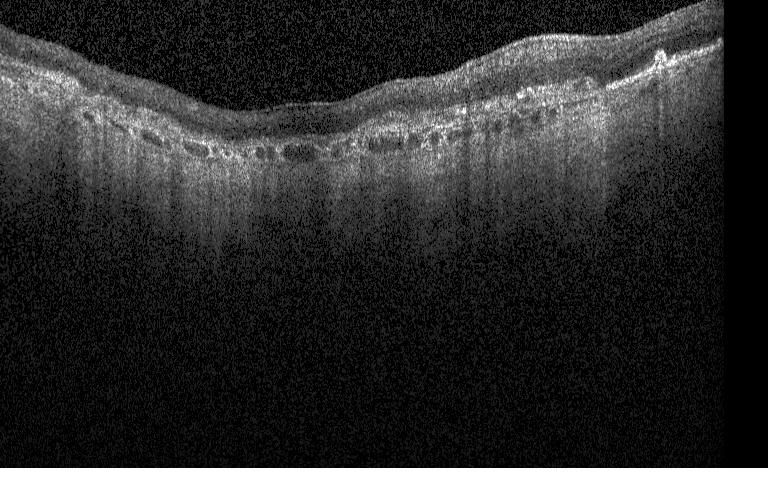
The scan shows a choroidal neovascular membrane.